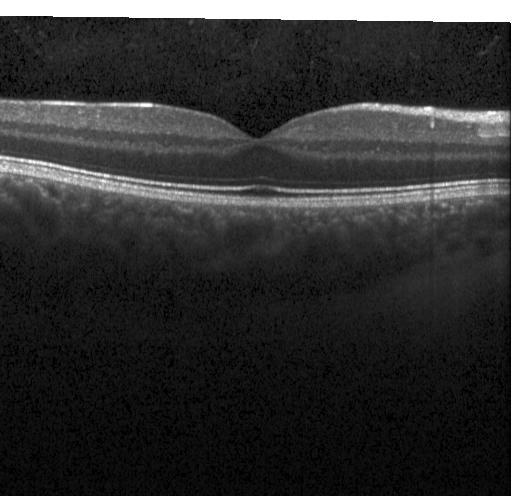
Dx: neither choroidal neovascularization, diabetic macular edema, nor drusen.